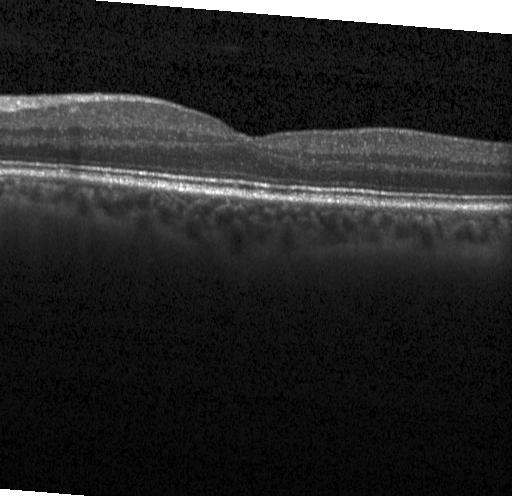 Instrument: Heidelberg Spectralis · SD-OCT · retinal OCT cross-section — Assessment: no evidence of CNV, DME, or drusen.